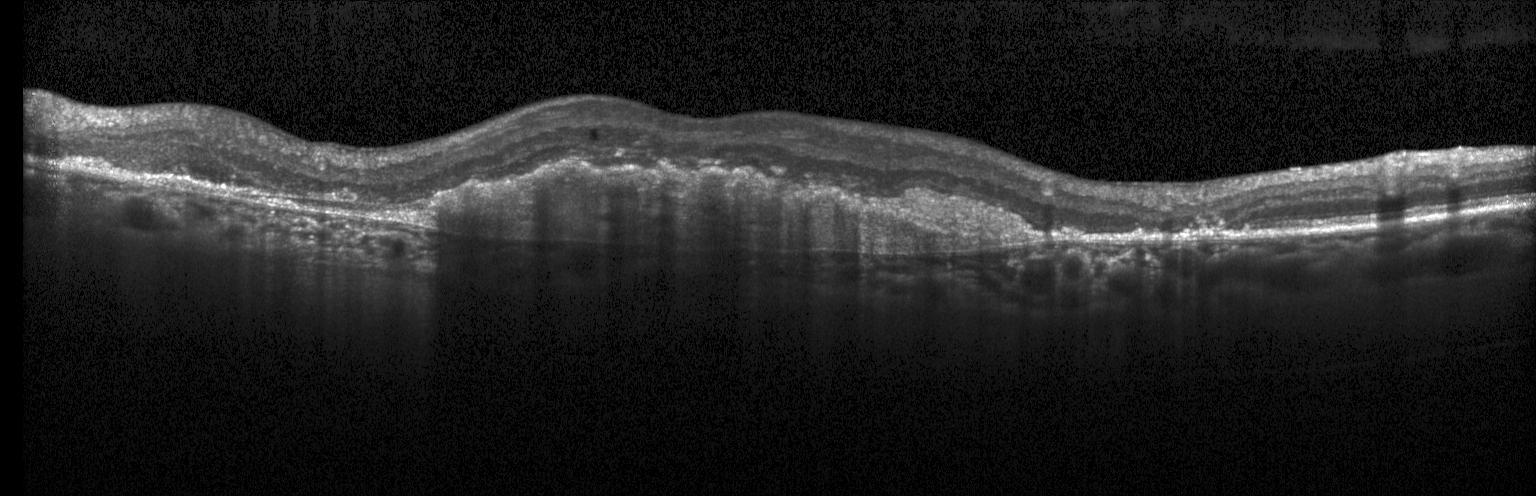
Macular OCT demonstrating a choroidal neovascular membrane.